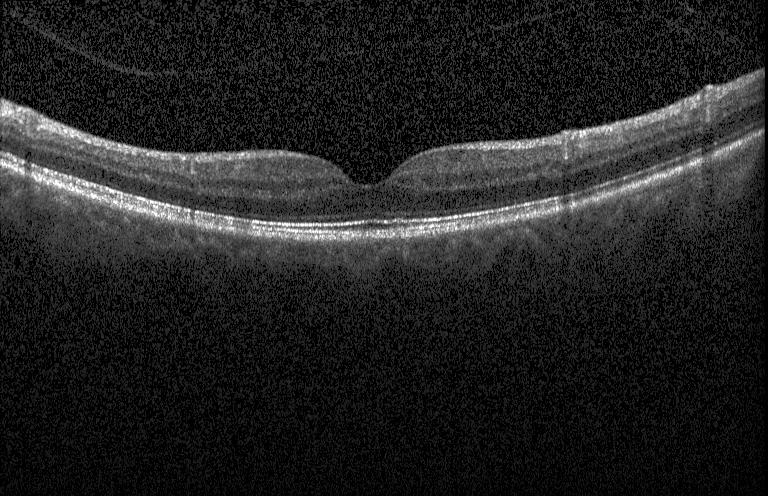 Centered on the fovea. Retinal OCT B-scan — Impression: neither choroidal neovascularization, diabetic macular edema, nor drusen.